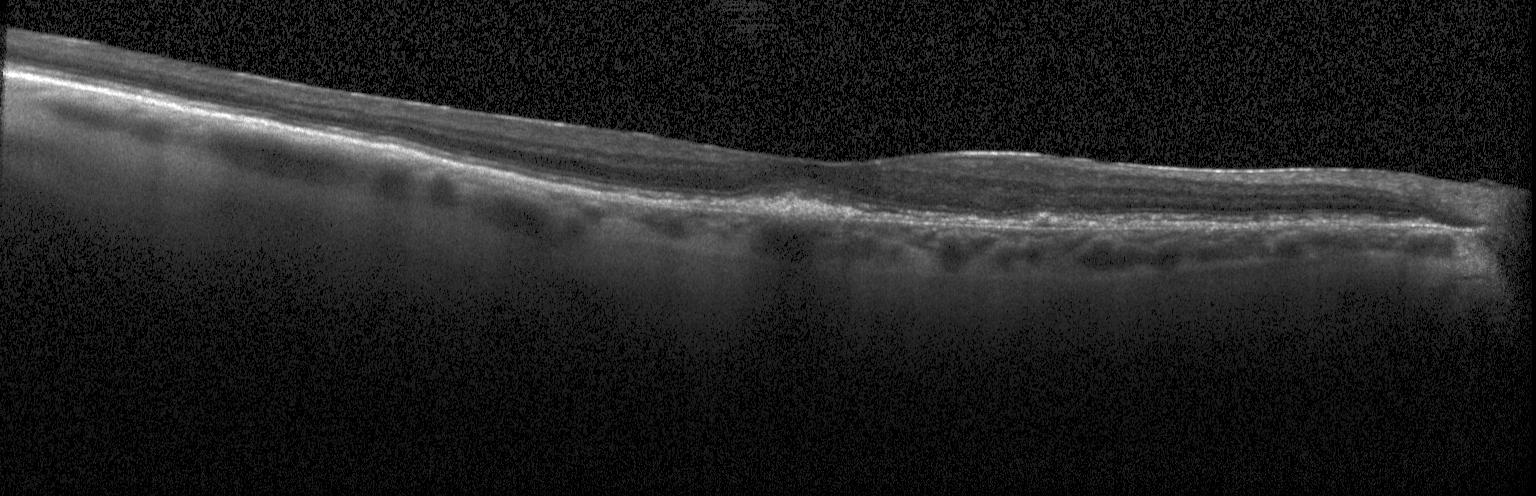
OCT B-scan
Finding: choroidal neovascularization.